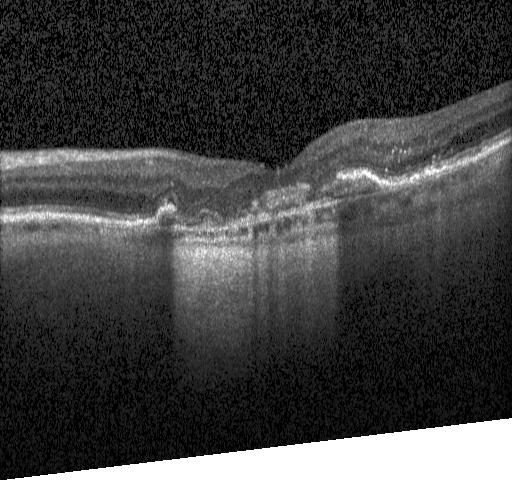

Diagnosis: choroidal neovascularization.